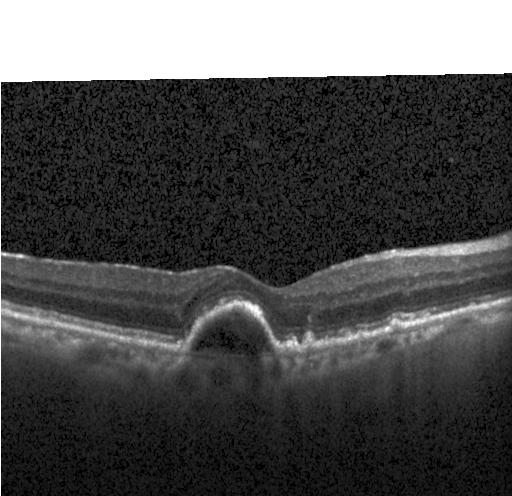

SD-OCT; optical coherence tomography scan. Finding: a choroidal neovascular membrane.